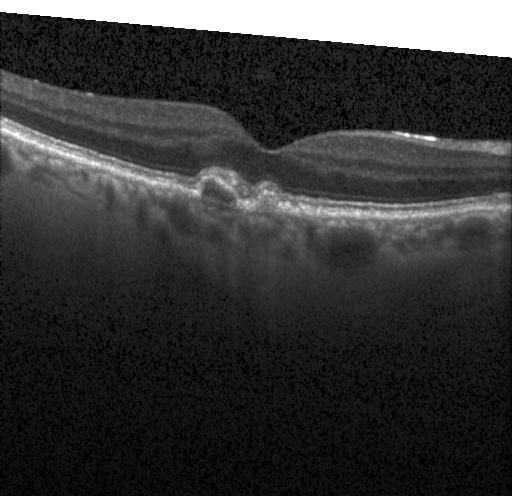 Optical coherence tomography scan
The scan shows CNV.